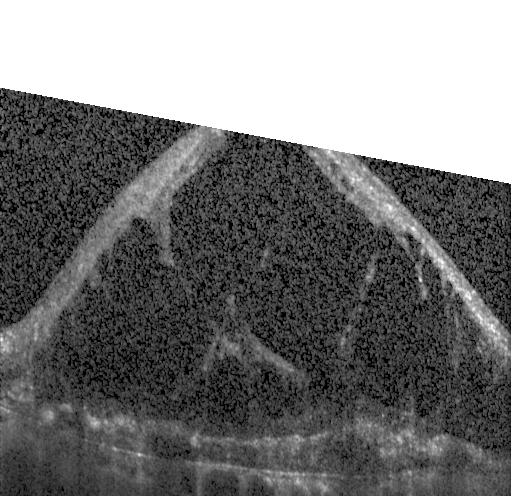 This B-scan demonstrates a choroidal neovascular membrane.